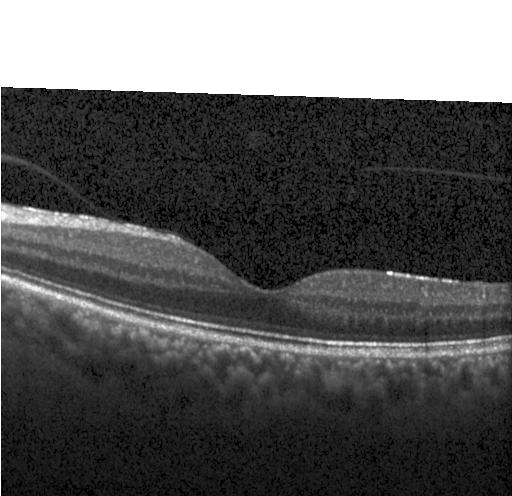

Optical coherence tomography scan. Spectral-domain OCT.
OCT finding: no evidence of CNV, DME, or drusen.